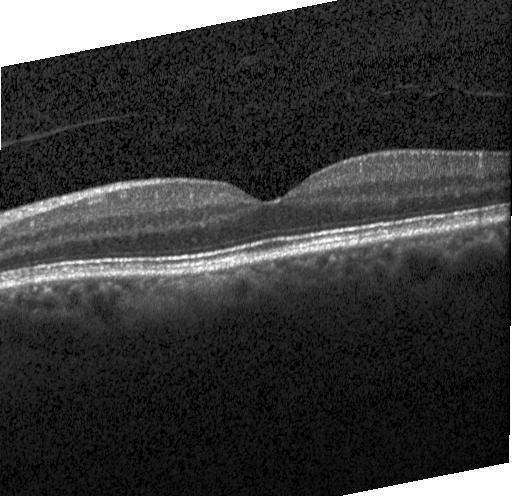 Heidelberg Spectralis OCT system, retinal OCT cross-section, spectral-domain optical coherence tomography, macular scan.
Diagnosis: no evidence of choroidal neovascularization, diabetic macular edema, or drusen.